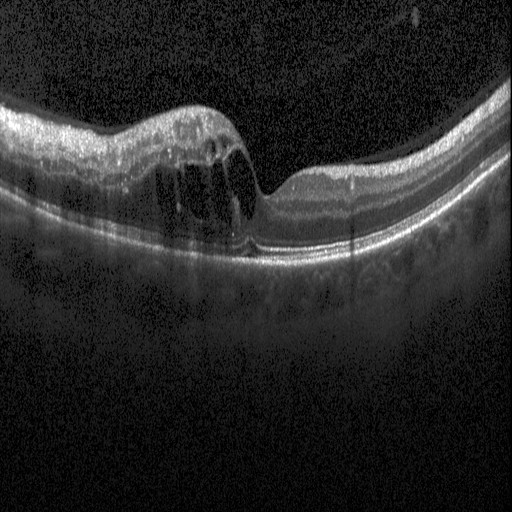
OCT B-scan showing diabetic macular edema (DME).